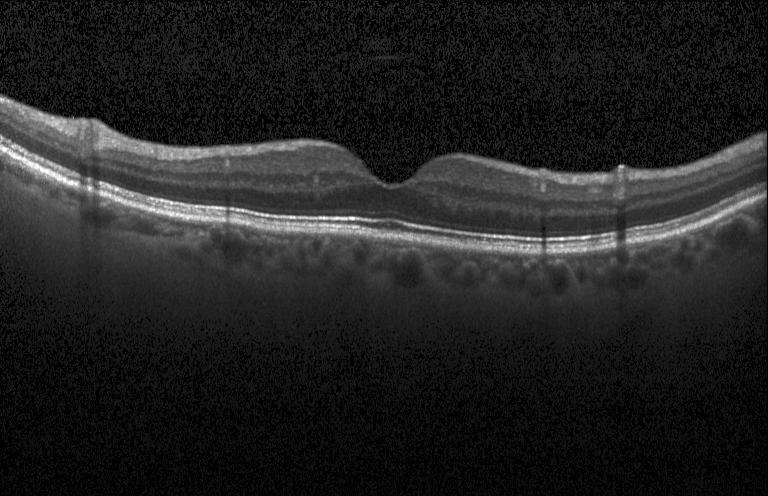

Spectral-domain OCT. Heidelberg Spectralis. Macular scan. Optical coherence tomography B-scan.
Diagnosis: no CNV, no DME, and no drusen.